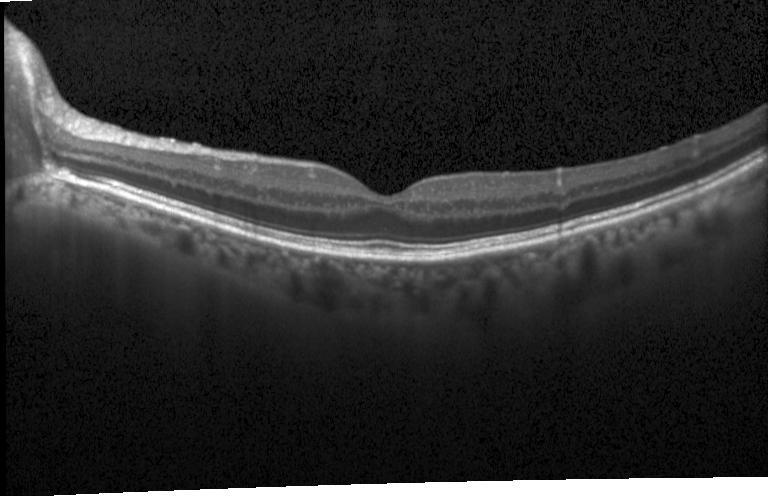 Diagnosis: no choroidal neovascularization, diabetic macular edema, or drusen.